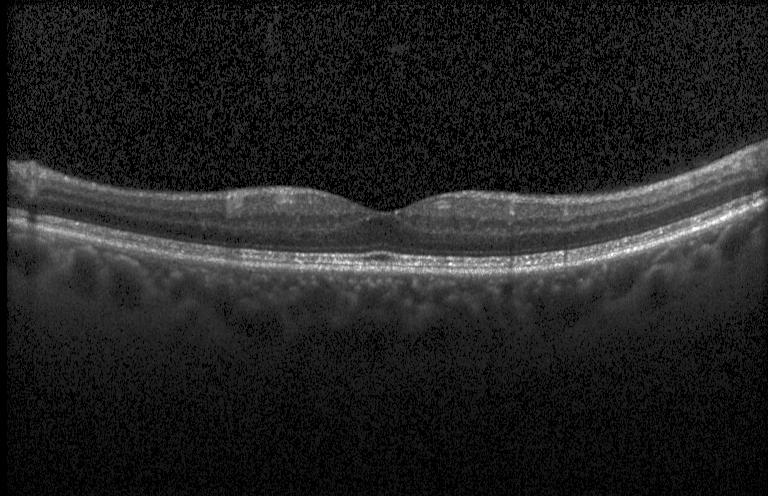 OCT B-scan, spectral-domain optical coherence tomography.
No choroidal neovascularization, no diabetic macular edema, and no drusen.